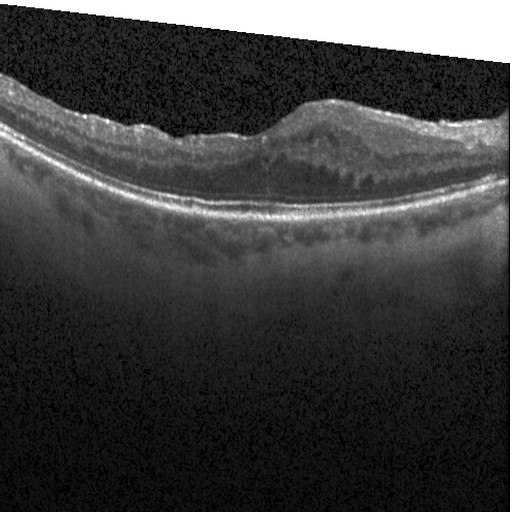 OCT line scan. DME.